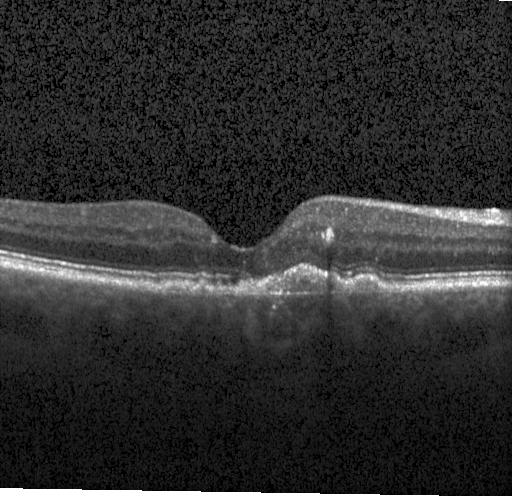 Impression: CNV.